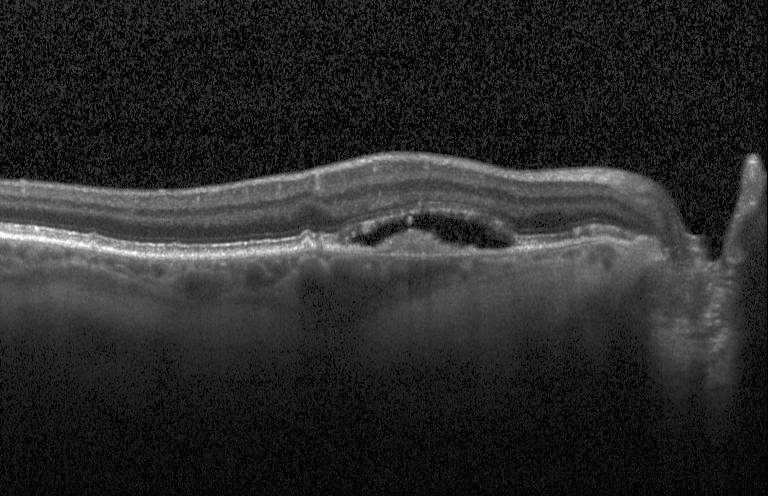
Retinal OCT B-scan · instrument: Heidelberg Spectralis.
Finding: a choroidal neovascular membrane.